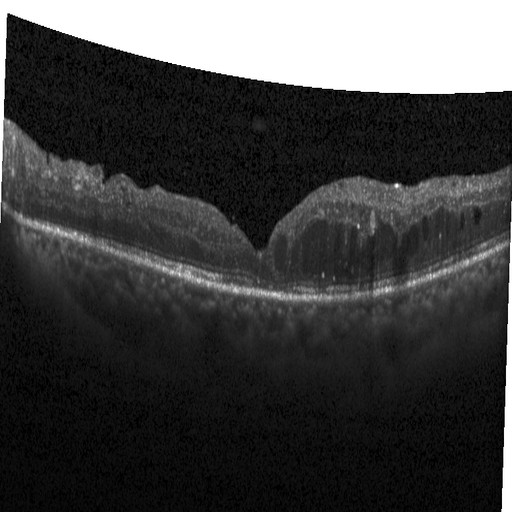 Heidelberg Spectralis OCT system. Retinal OCT B-scan
OCT finding: DME.